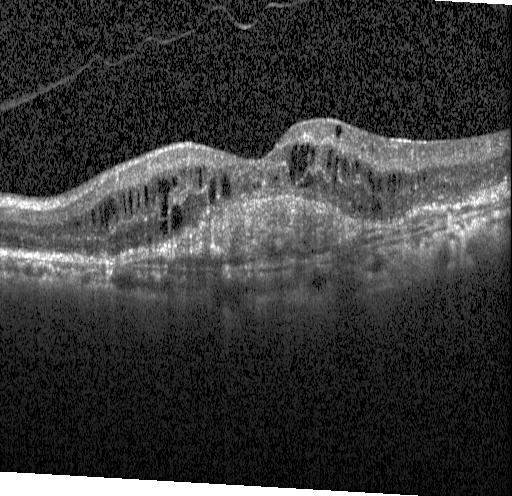

Heidelberg Spectralis OCT system, retinal OCT B-scan, macular scan, spectral-domain optical coherence tomography. The scan shows choroidal neovascularization (CNV).